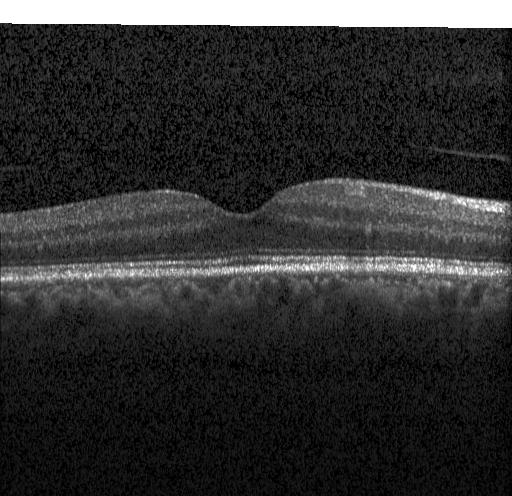

Fovea-centered; retinal OCT cross-section — Assessment: no choroidal neovascularization, no diabetic macular edema, and no drusen.